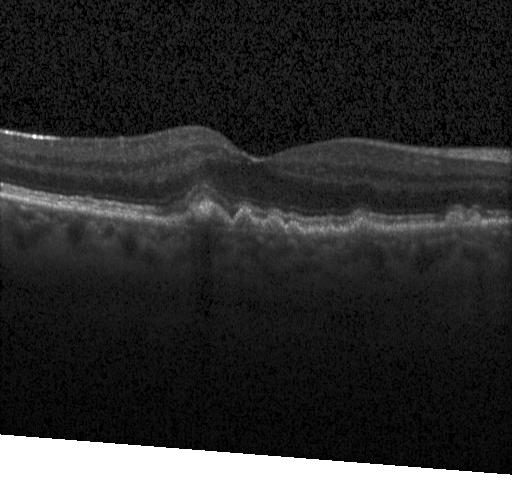 Diagnosis: sub-RPE drusenoid deposits.